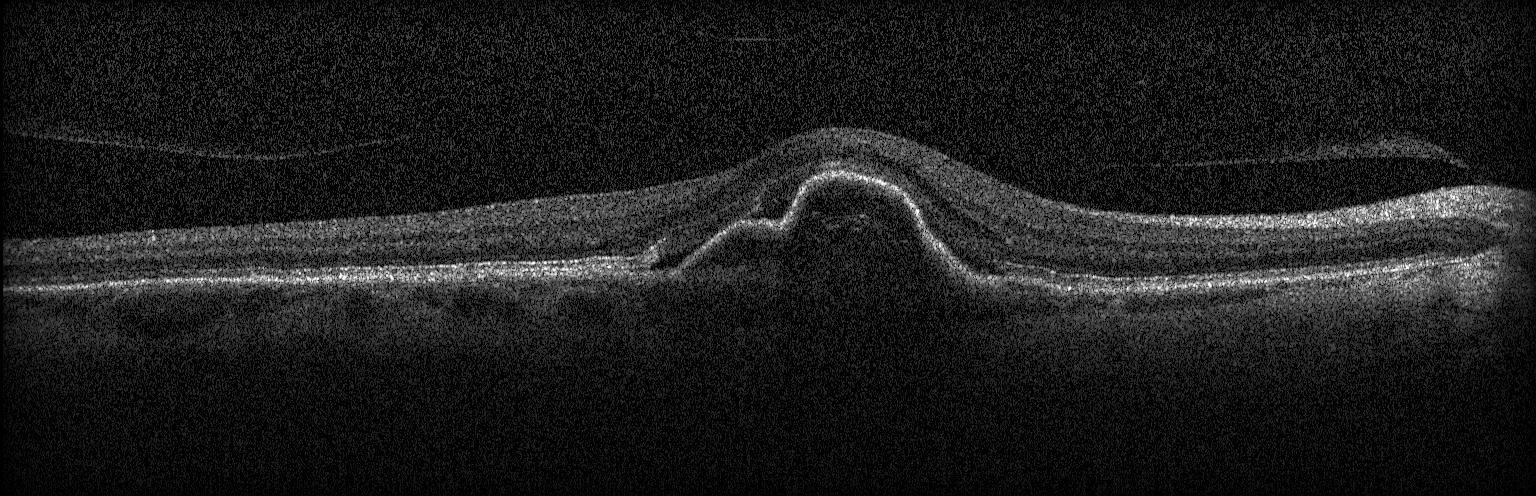
Retinal OCT B-scan. Macular scan
Diagnosis: a choroidal neovascular membrane.